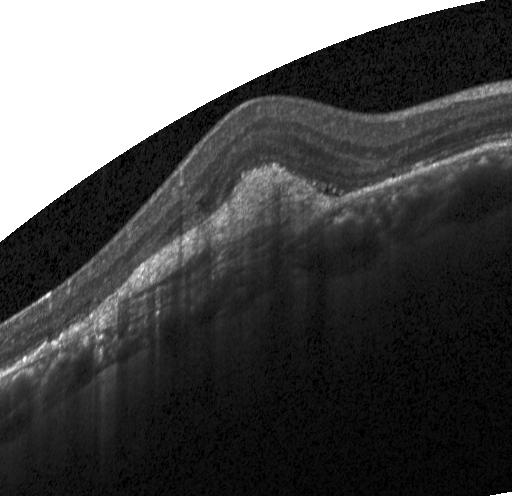

Horizontal scan through the fovea, OCT line scan, spectral-domain OCT, acquired on a Heidelberg Spectralis. Finding: a choroidal neovascular membrane.